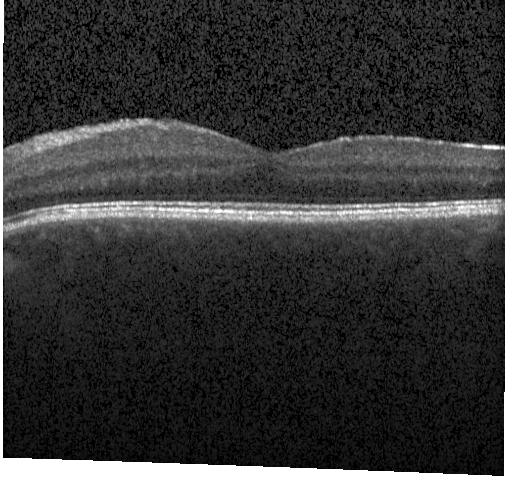

Heidelberg Spectralis · through the macula · spectral-domain optical coherence tomography · retinal OCT cross-section
Macular OCT: no evidence of choroidal neovascularization, diabetic macular edema, or drusen.